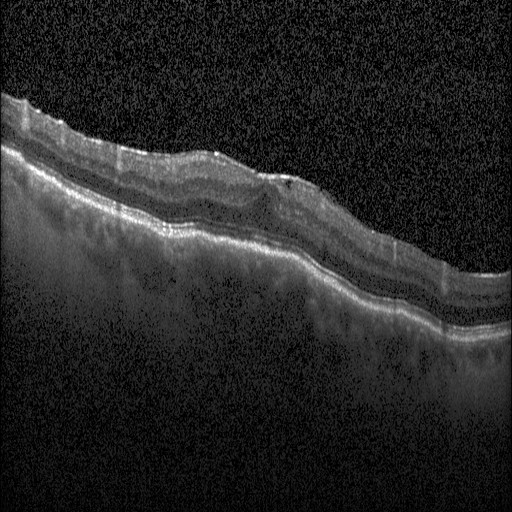 Macular OCT demonstrating diabetic macular edema.